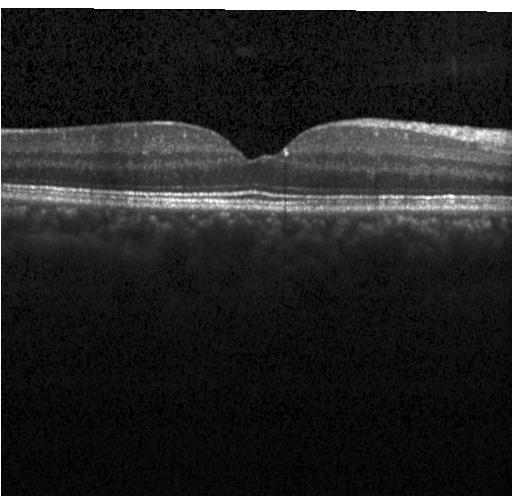
SD-OCT. Retinal OCT cross-section. Centered on the fovea. No choroidal neovascularization, diabetic macular edema, or drusen.